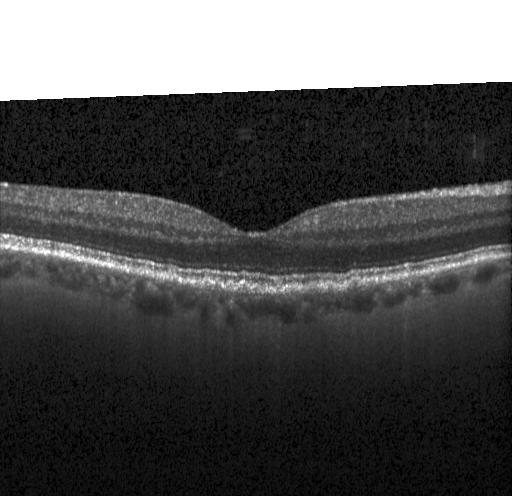
Centered on the fovea. Retinal OCT cross-section.
Dx: sub-RPE drusenoid deposits.